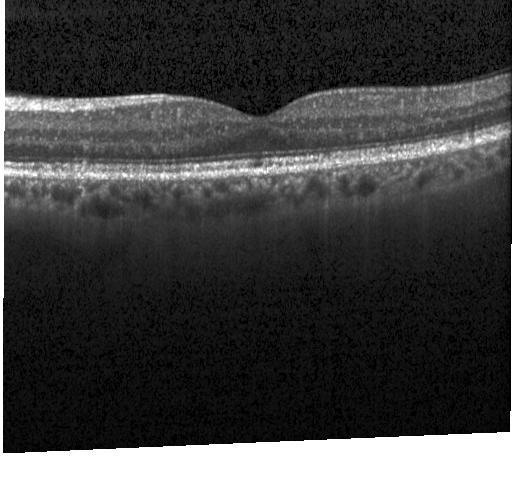 Heidelberg Spectralis OCT system; spectral-domain OCT; optical coherence tomography scan; centered on the fovea
The scan shows no CNV, DME, or drusen.